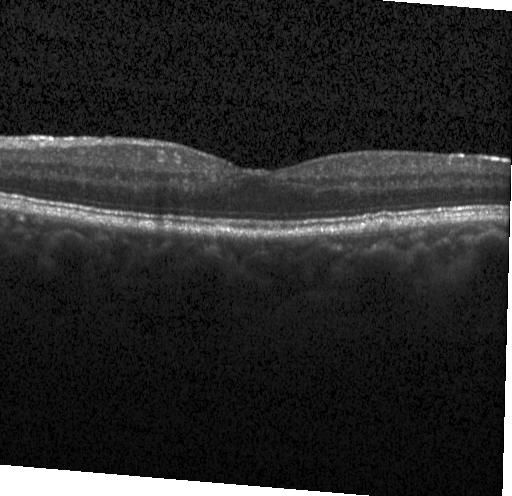
OCT line scan
Impression: multiple drusen.